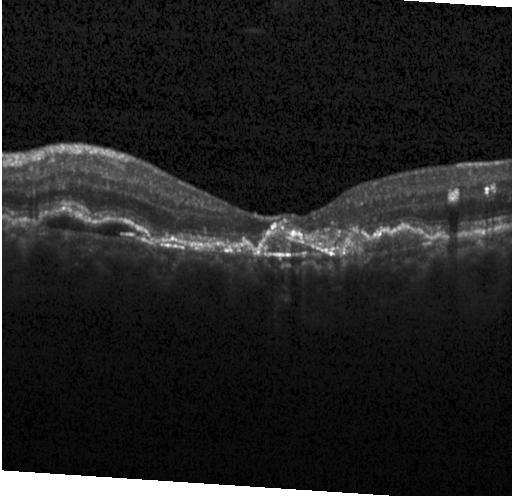
Centered on the fovea, OCT B-scan, acquired on a Heidelberg Spectralis, SD-OCT — The scan shows a choroidal neovascular membrane.